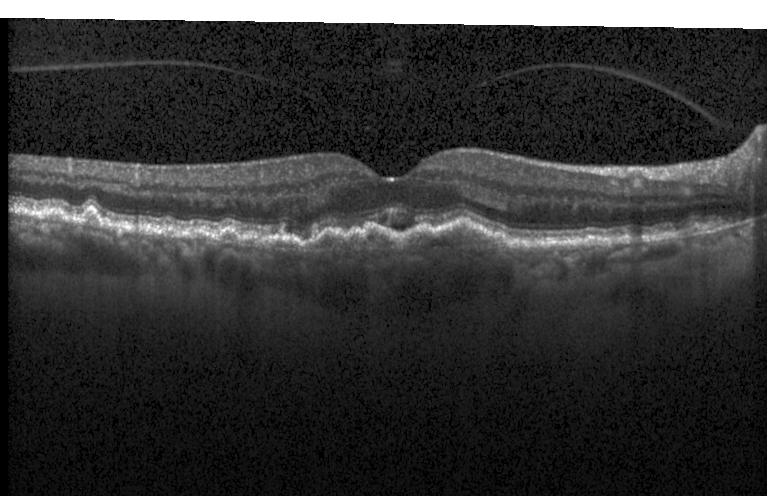

Through the macula; retinal OCT B-scan; Heidelberg Spectralis OCT system
Impression: a choroidal neovascular membrane.